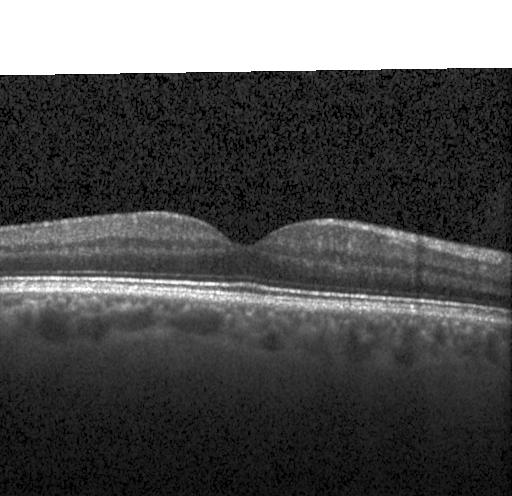
Optical coherence tomography B-scan
This B-scan demonstrates no evidence of choroidal neovascularization, diabetic macular edema, or drusen.